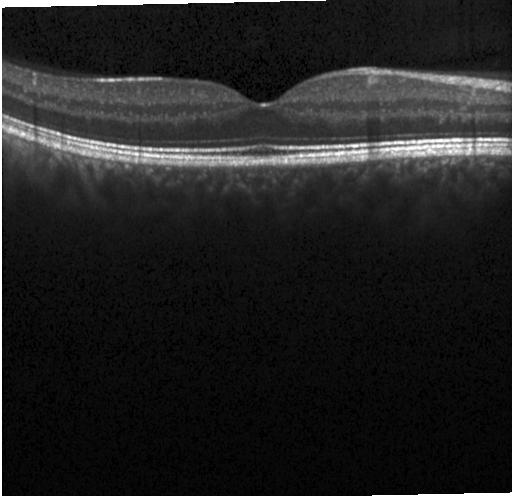

SD-OCT · optical coherence tomography scan · acquired on a Heidelberg Spectralis
Diagnosis: no choroidal neovascularization, no diabetic macular edema, and no drusen.